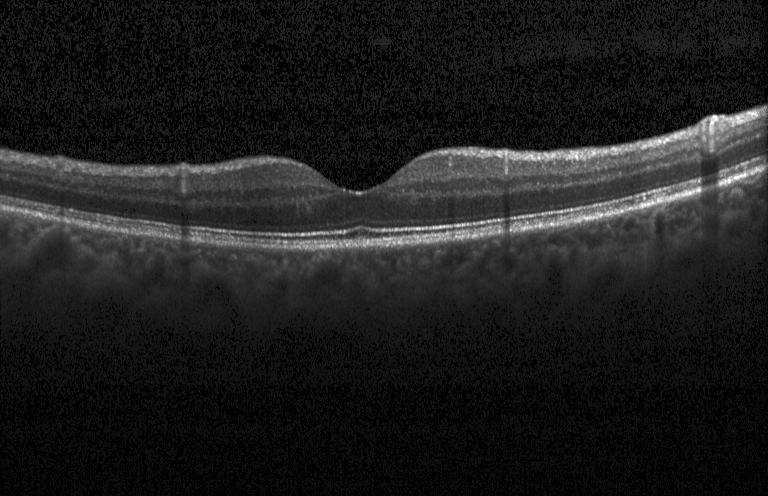 Optical coherence tomography B-scan, macular scan.
Diagnosis: neither CNV, DME, nor drusen.